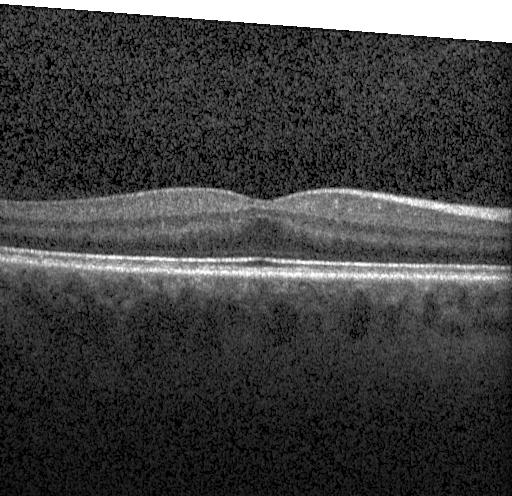
Optical coherence tomography scan. Assessment: no CNV, DME, or drusen.